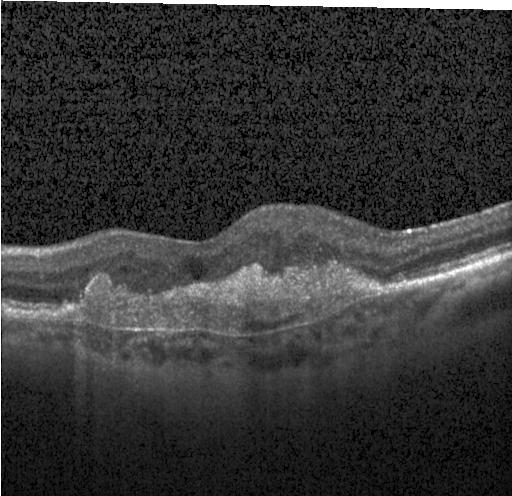
OCT scan showing a choroidal neovascular membrane.